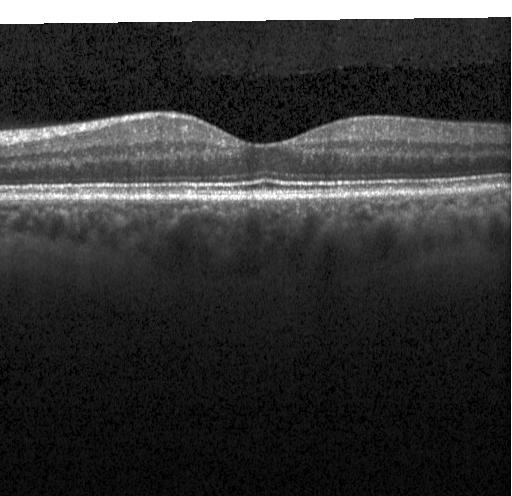 This B-scan demonstrates no choroidal neovascularization, no diabetic macular edema, and no drusen.